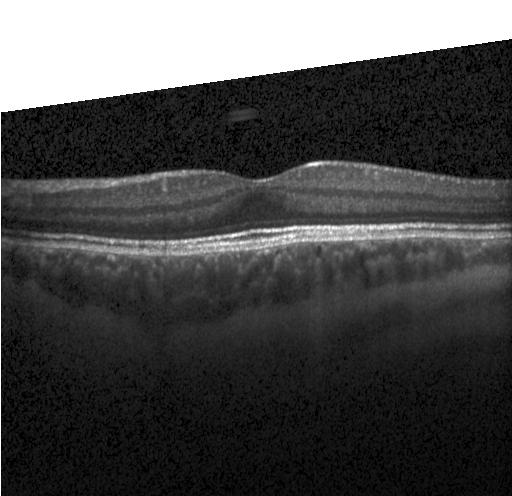 Macular OCT: no CNV, no DME, and no drusen.